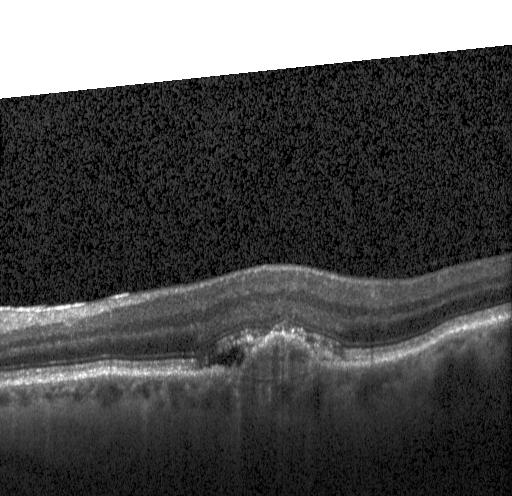 Centered on the fovea, OCT line scan
This B-scan demonstrates a choroidal neovascular membrane.